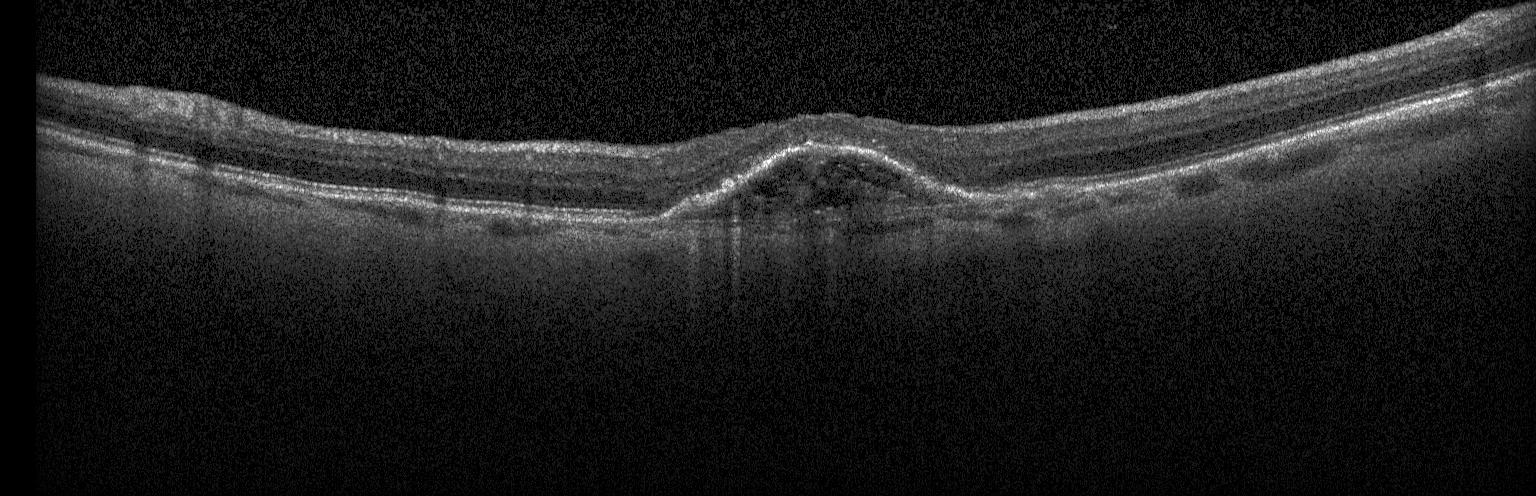 Dx: a choroidal neovascular membrane.